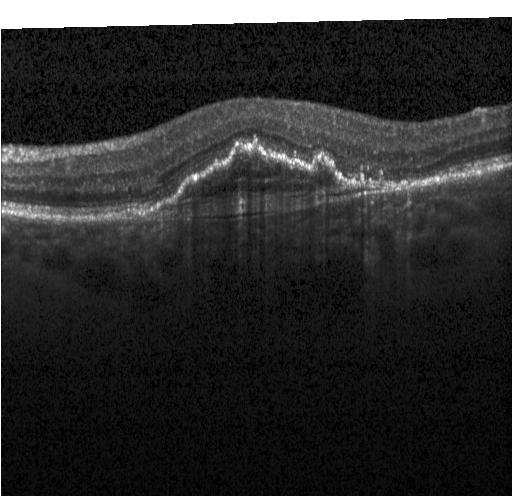
A choroidal neovascular membrane.